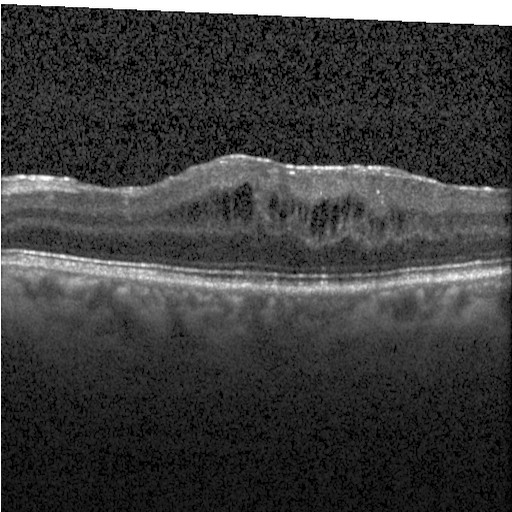 Retinal OCT B-scan; SD-OCT; horizontal scan through the fovea — Macular OCT: diabetic macular edema (DME).